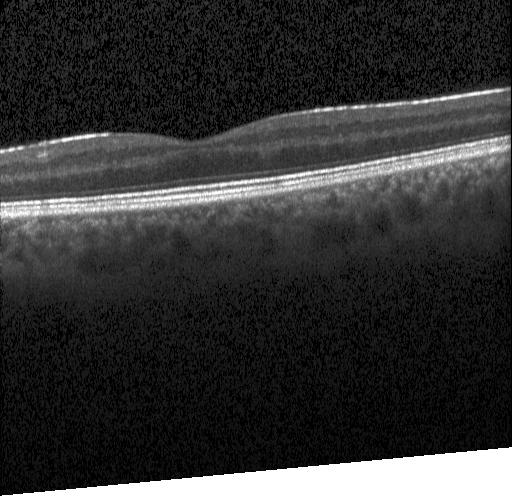 OCT B-scan, acquired on a Heidelberg Spectralis, centered on the fovea
Diagnosis: no choroidal neovascularization, no diabetic macular edema, and no drusen.